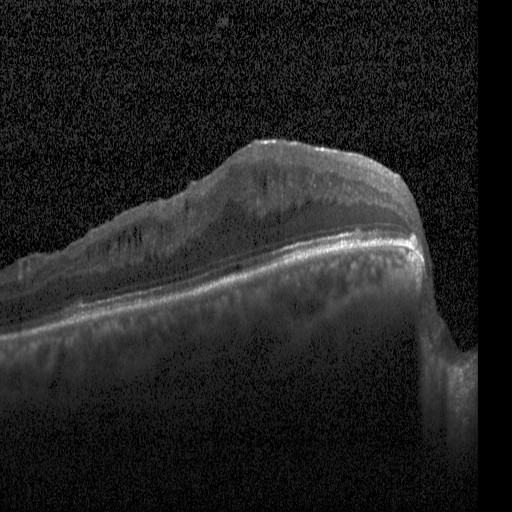 Dx: diabetic macular edema.